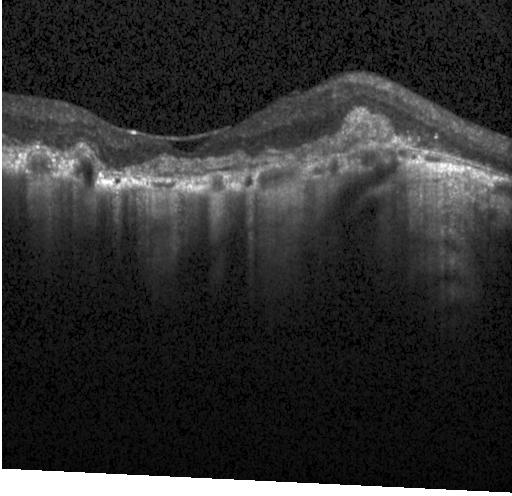

OCT line scan; acquired on a Heidelberg Spectralis; macular scan.
This B-scan demonstrates choroidal neovascularization.